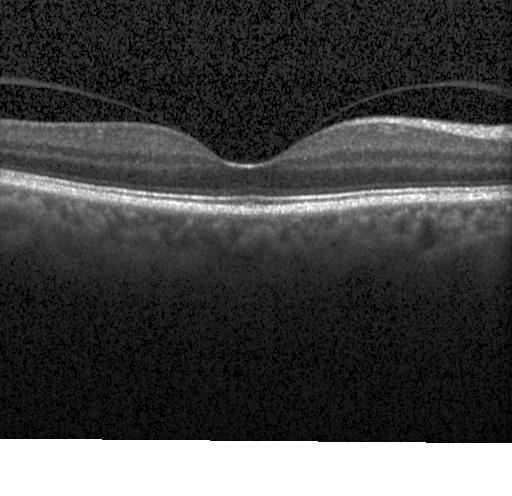

Optical coherence tomography B-scan
Assessment: no evidence of choroidal neovascularization, diabetic macular edema, or drusen.